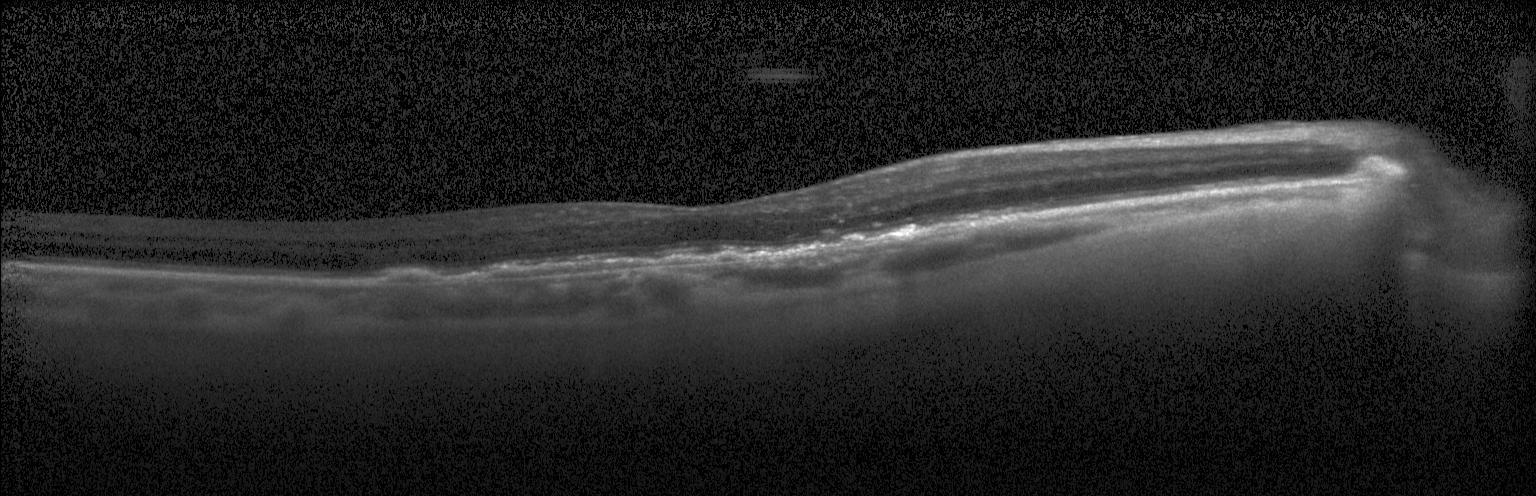
Retinal OCT B-scan. Centered on the fovea. Dx: choroidal neovascularization (CNV).